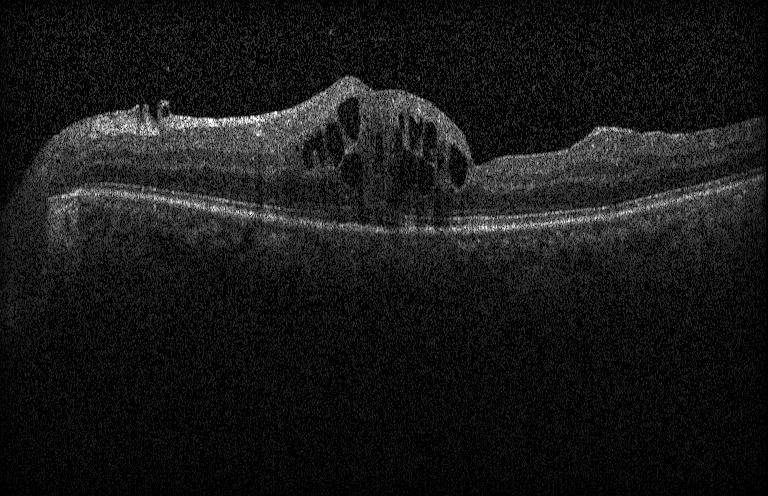
Heidelberg Spectralis OCT system, centered on the fovea, spectral-domain optical coherence tomography, optical coherence tomography scan
Dx: DME.